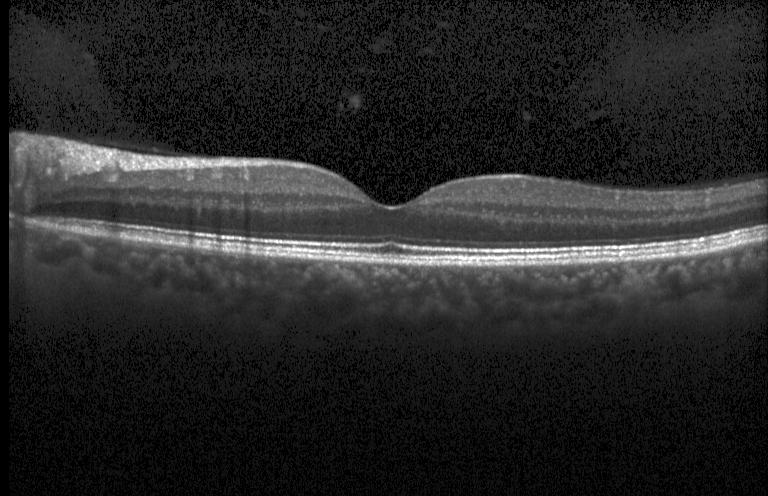

SD-OCT; through the macula; acquired on a Heidelberg Spectralis; OCT line scan — This B-scan demonstrates no CNV, DME, or drusen.